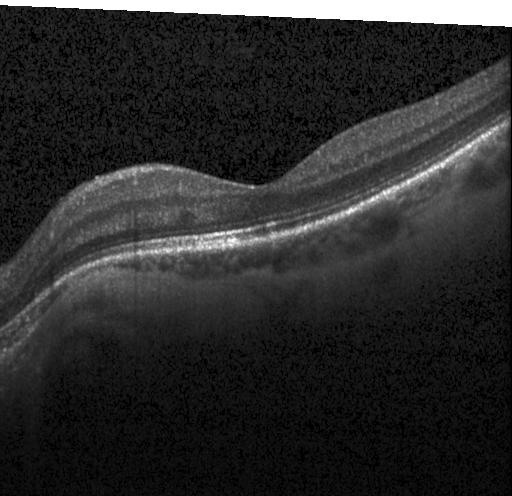
Dx: no evidence of choroidal neovascularization, diabetic macular edema, or drusen.